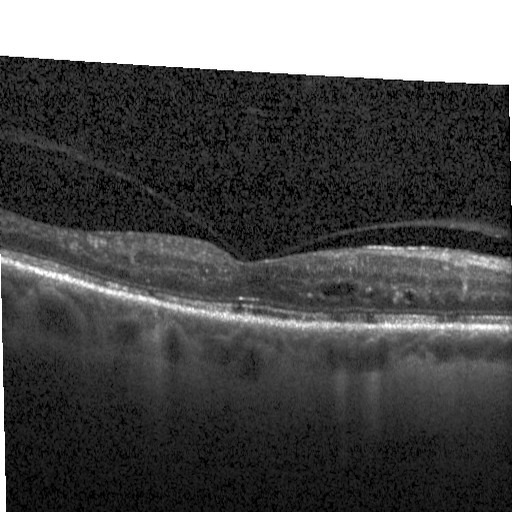

Heidelberg Spectralis OCT system. Spectral-domain OCT. Fovea-centered. OCT B-scan.
Finding: diabetic macular edema.